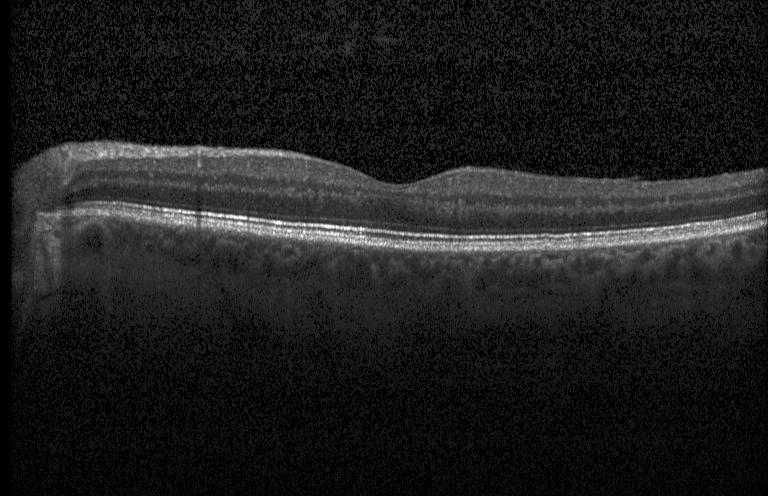 Optical coherence tomography B-scan, centered on the fovea, spectral-domain OCT — Assessment: no CNV, DME, or drusen.